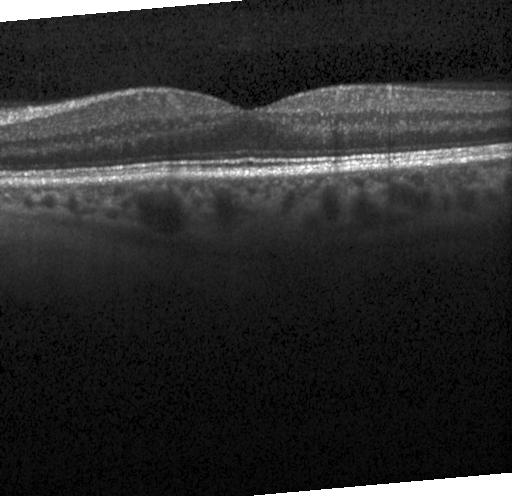 Impression: no choroidal neovascularization, diabetic macular edema, or drusen.